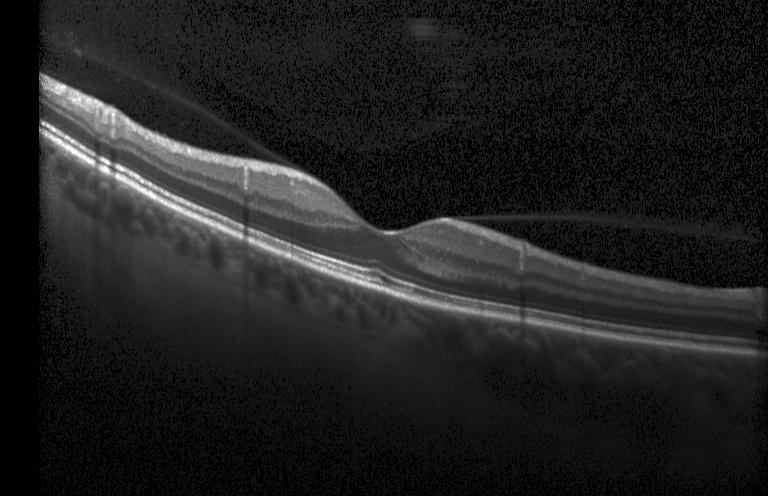 Finding: no evidence of choroidal neovascularization, diabetic macular edema, or drusen.